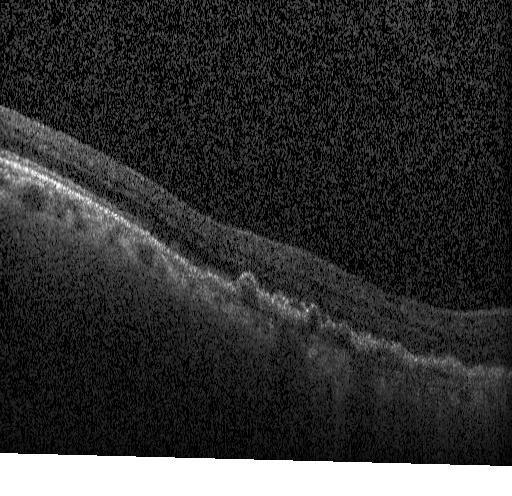

Retinal OCT cross-section; spectral-domain OCT; acquired on a Heidelberg Spectralis; fovea-centered
Diagnosis: a choroidal neovascular membrane.